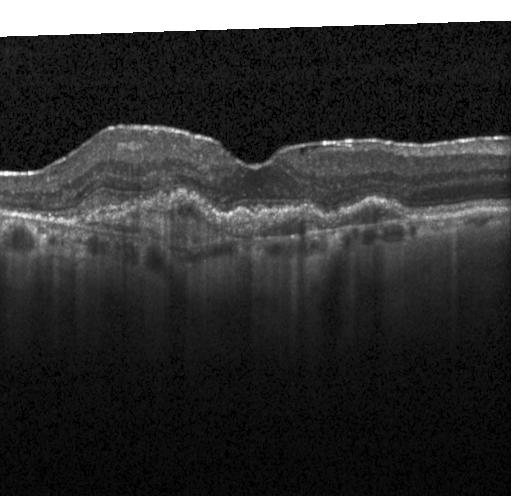
OCT B-scan; Heidelberg Spectralis OCT system; through the macula; SD-OCT — The scan shows choroidal neovascularization.